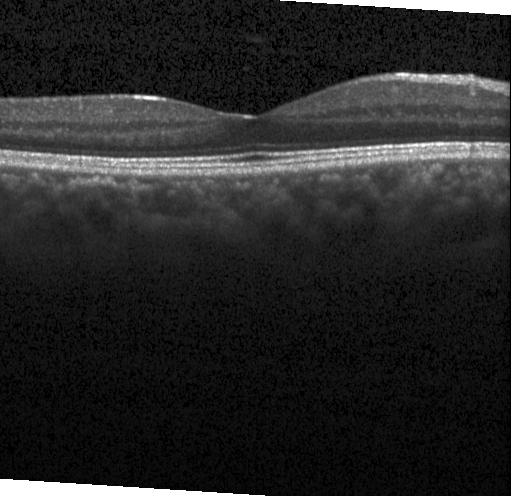

SD-OCT. OCT B-scan. The scan shows no evidence of CNV, DME, or drusen.